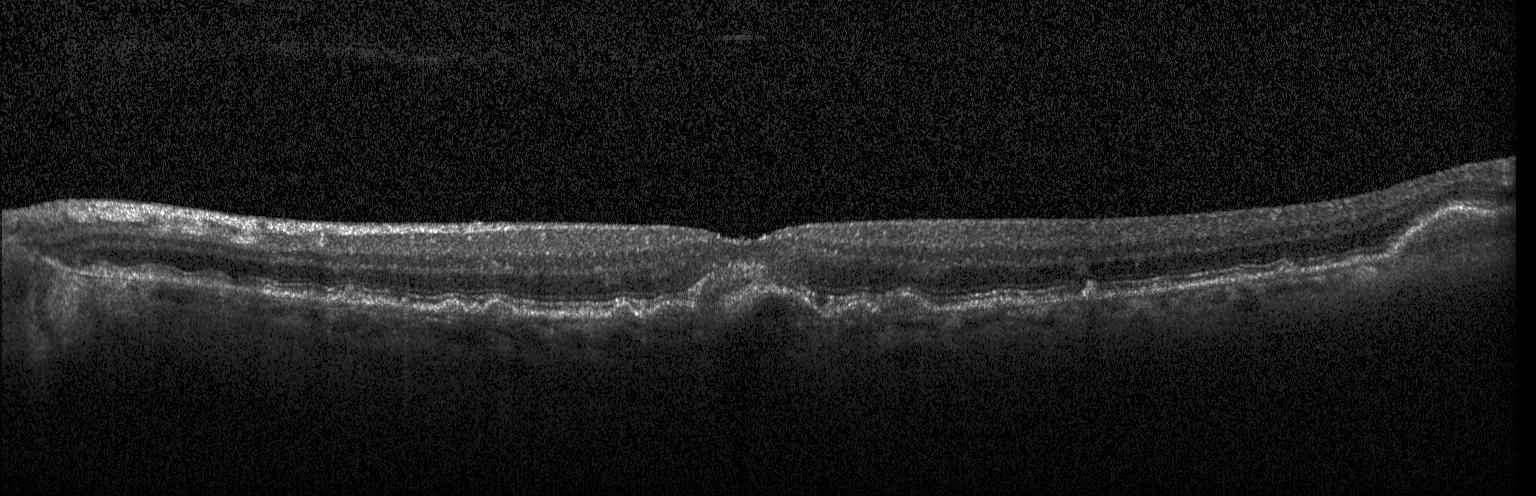
Acquired on a Heidelberg Spectralis, horizontal scan through the fovea, OCT B-scan. Finding: a choroidal neovascular membrane.